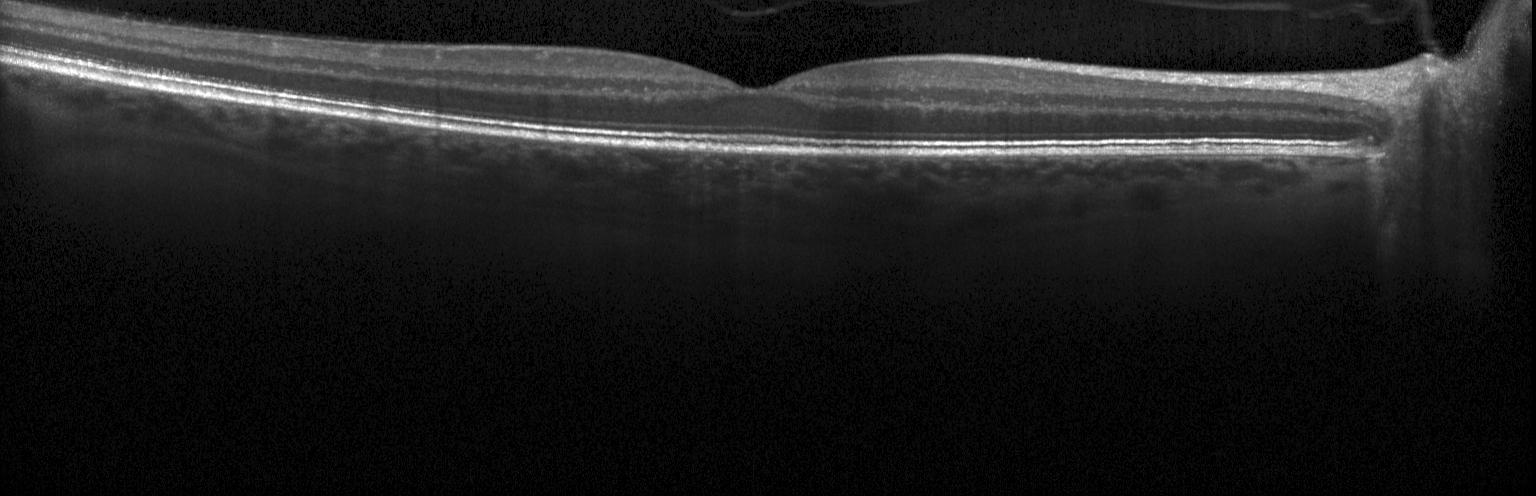 Retinal OCT B-scan. Macular scan — Impression: neither choroidal neovascularization, diabetic macular edema, nor drusen.